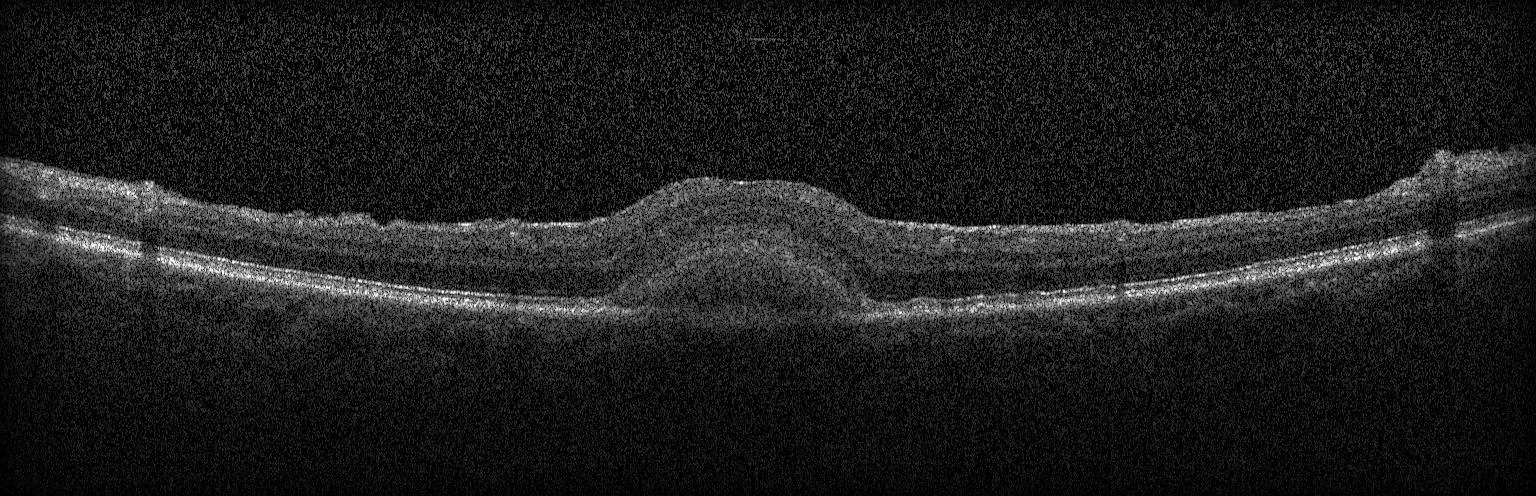
Horizontal scan through the fovea; Heidelberg Spectralis OCT system; spectral-domain OCT; optical coherence tomography B-scan
Impression: a choroidal neovascular membrane.